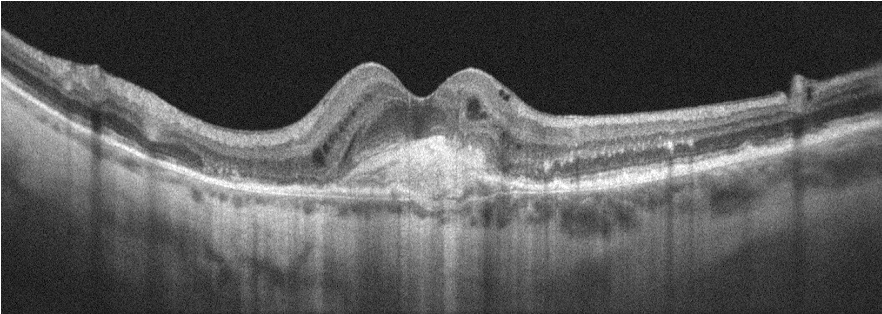

Diagnosis: AMD.